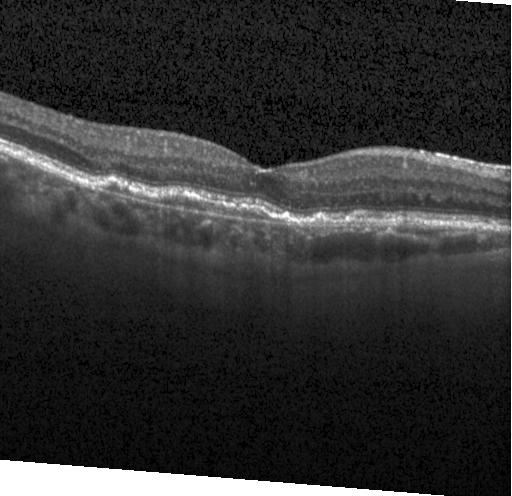

Retinal OCT cross-section
Impression: a choroidal neovascular membrane.